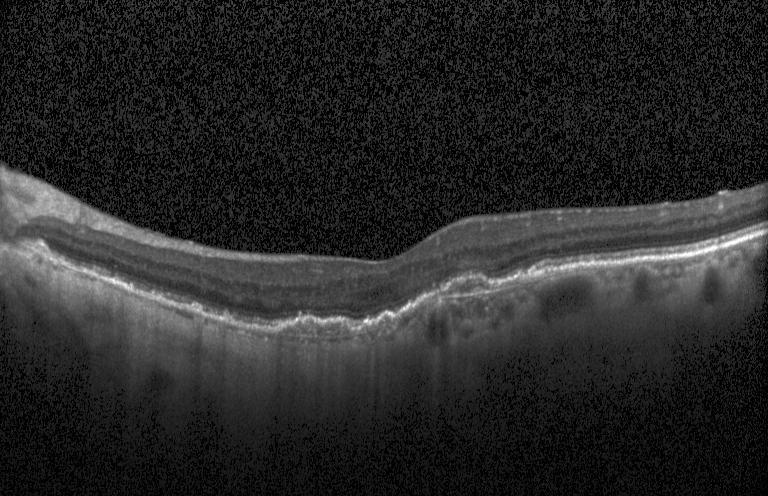

Finding: choroidal neovascularization (CNV).